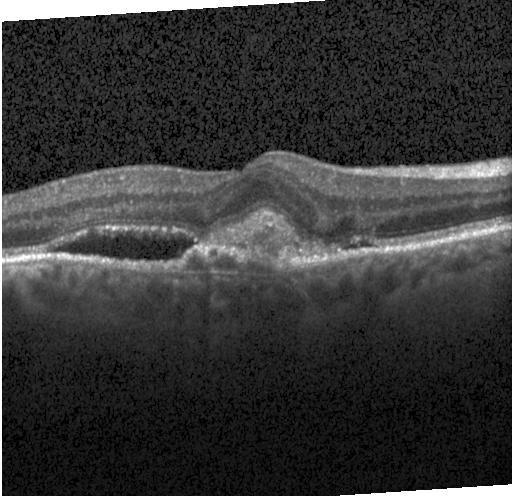
Diagnosis: a choroidal neovascular membrane.